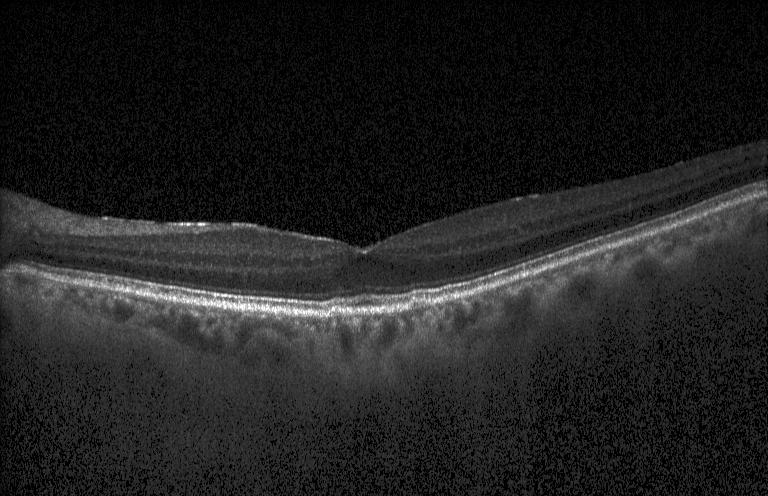
Retinal OCT cross-section, Heidelberg Spectralis OCT system, through the macula, spectral-domain OCT.
Multiple drusen.